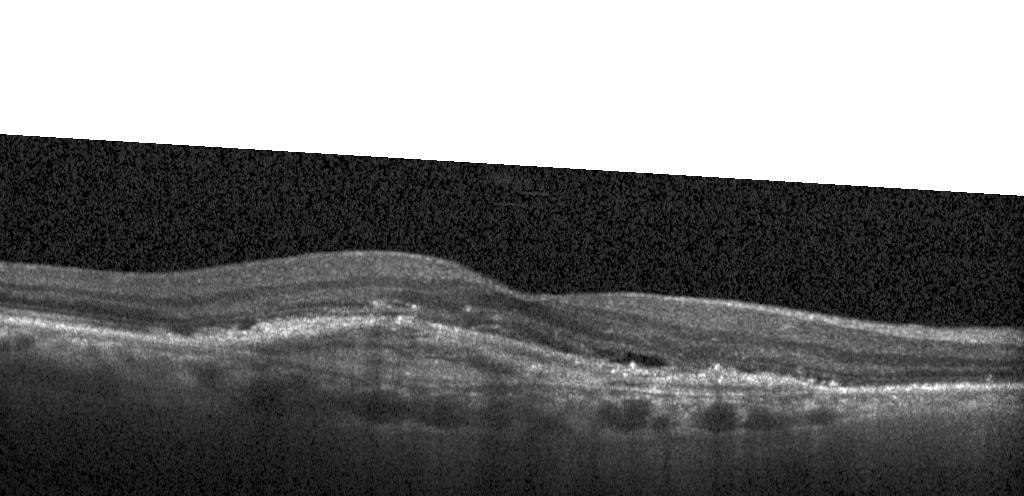
OCT B-scan; horizontal scan through the fovea; spectral-domain optical coherence tomography; Heidelberg Spectralis
Assessment: a choroidal neovascular membrane.